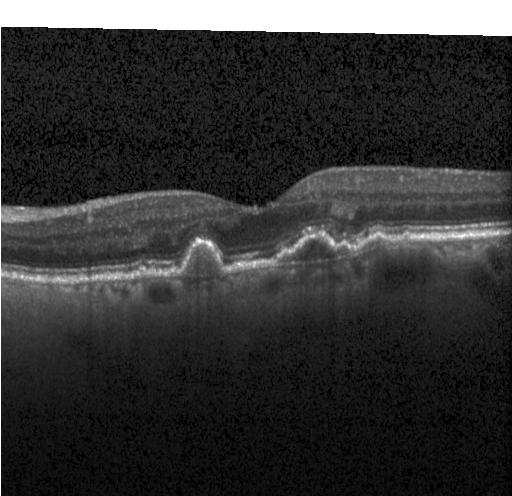

SD-OCT; optical coherence tomography B-scan.
Impression: a choroidal neovascular membrane.